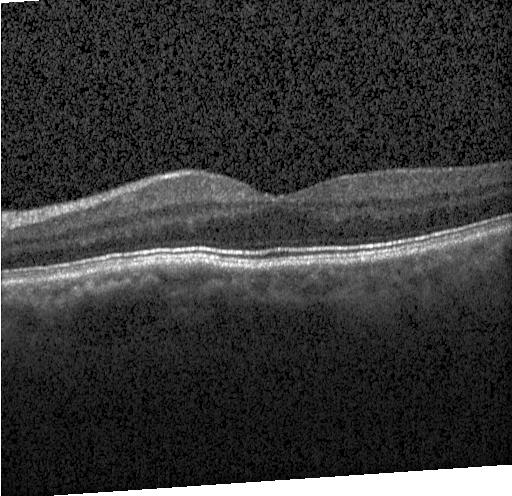 Retinal OCT B-scan · Heidelberg Spectralis OCT system · spectral-domain OCT.
Finding: no choroidal neovascularization, diabetic macular edema, or drusen.